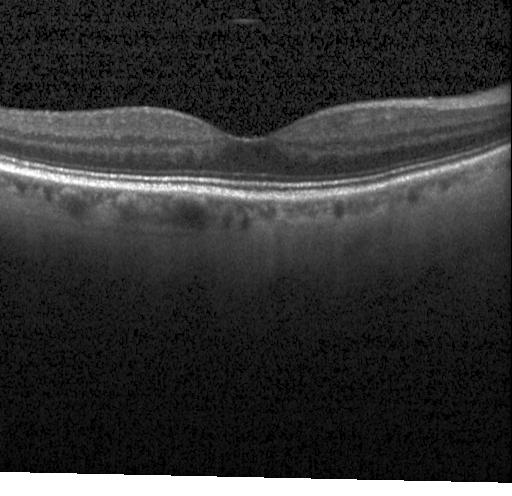

Instrument: Heidelberg Spectralis · spectral-domain optical coherence tomography · optical coherence tomography B-scan. Finding: no CNV, no DME, and no drusen.